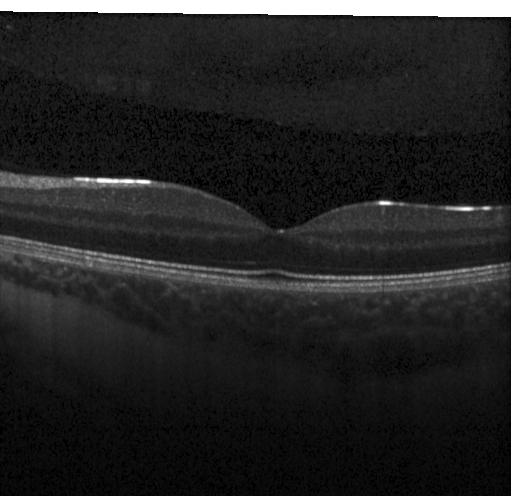 Optical coherence tomography scan; through the macula; spectral-domain optical coherence tomography; Heidelberg Spectralis.
Diagnosis: neither choroidal neovascularization, diabetic macular edema, nor drusen.